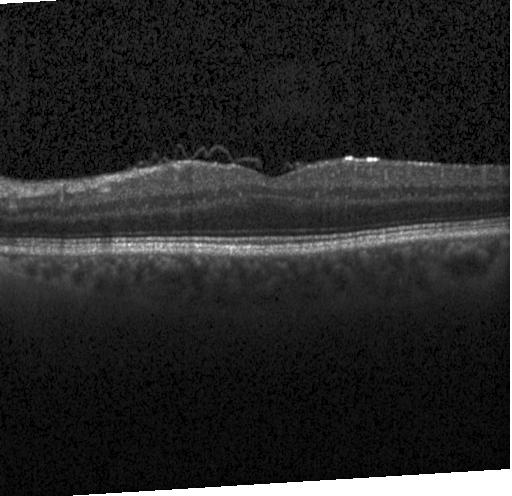

Heidelberg Spectralis OCT system; retinal OCT B-scan.
Impression: no CNV, DME, or drusen.